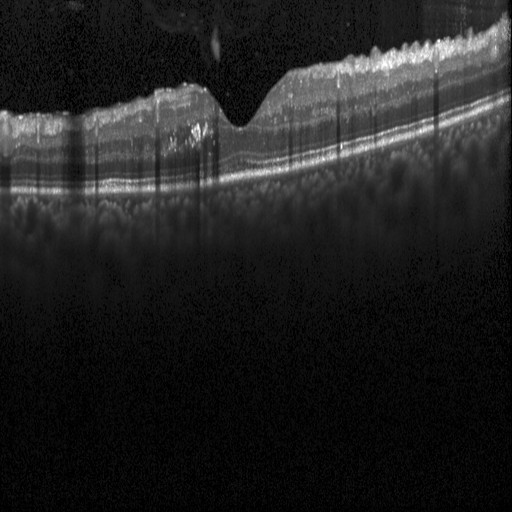 Impression: diabetic macular edema.